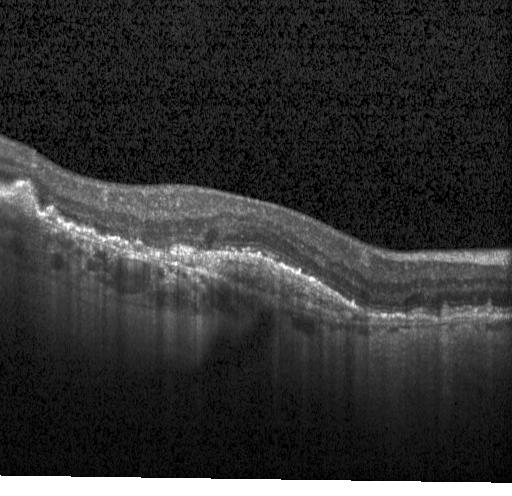
Centered on the fovea, retinal OCT cross-section, acquired on a Heidelberg Spectralis, spectral-domain optical coherence tomography.
Finding: a choroidal neovascular membrane.